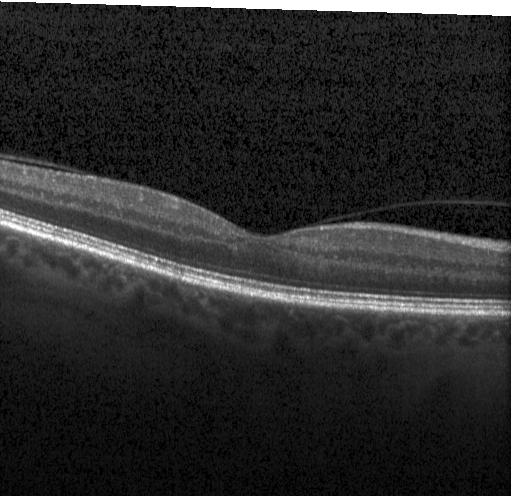 Retinal OCT cross-section · through the macula. Diagnosis: no choroidal neovascularization, no diabetic macular edema, and no drusen.